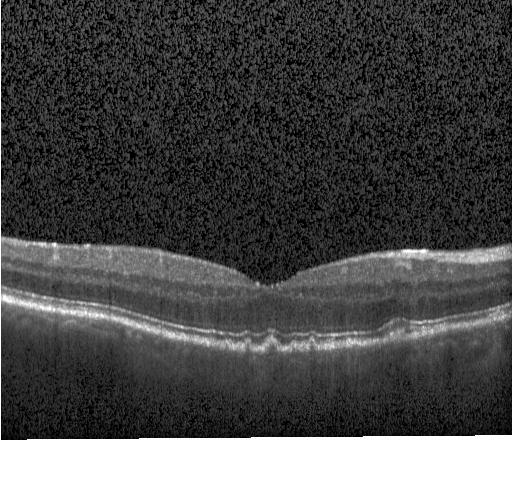

SD-OCT · retinal OCT B-scan · instrument: Heidelberg Spectralis — Sub-RPE drusenoid deposits.